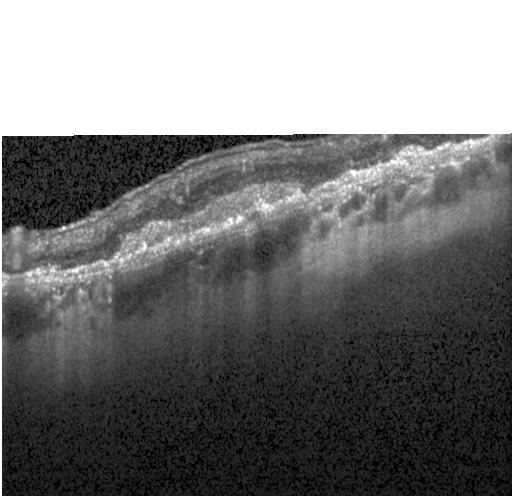 This B-scan demonstrates a choroidal neovascular membrane.